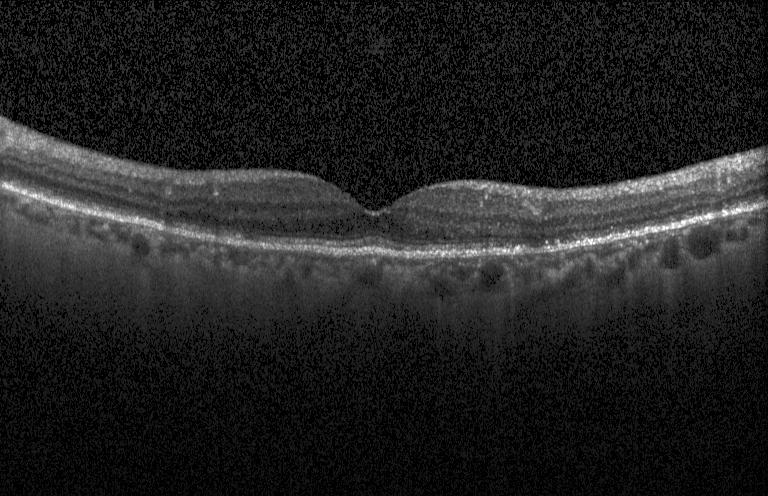 Macular OCT demonstrating no choroidal neovascularization, diabetic macular edema, or drusen.